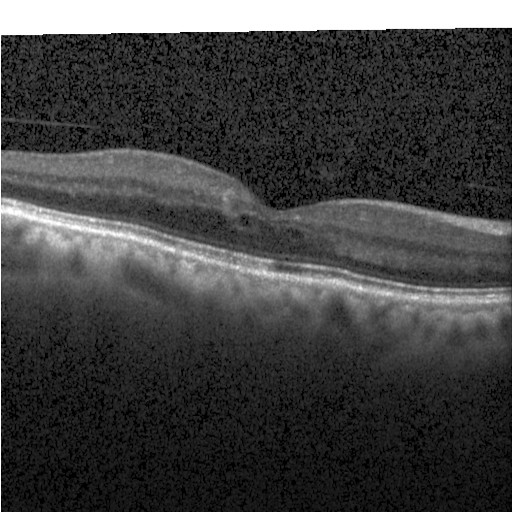

Macular OCT demonstrating diabetic macular edema.